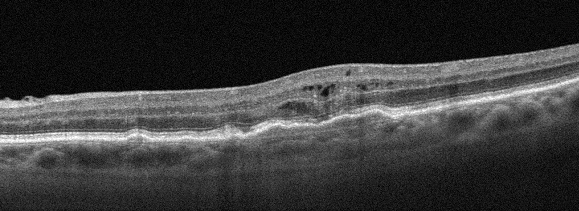 Oculus sinister. Acquired on an Optovue Avanti RTVue XR. Retinal OCT B-scan.
Diagnosis: age-related macular degeneration (AMD).